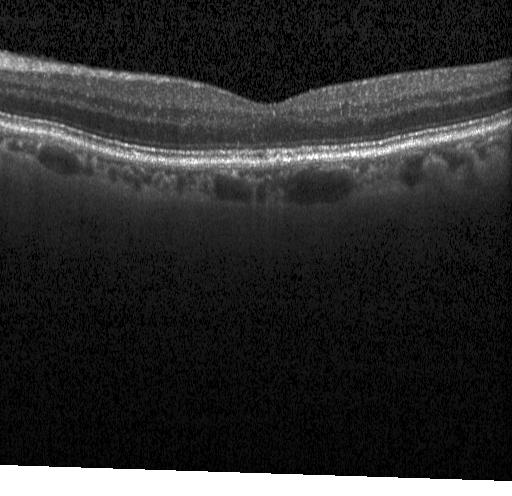
Retinal OCT cross-section
The scan shows no choroidal neovascularization, diabetic macular edema, or drusen.